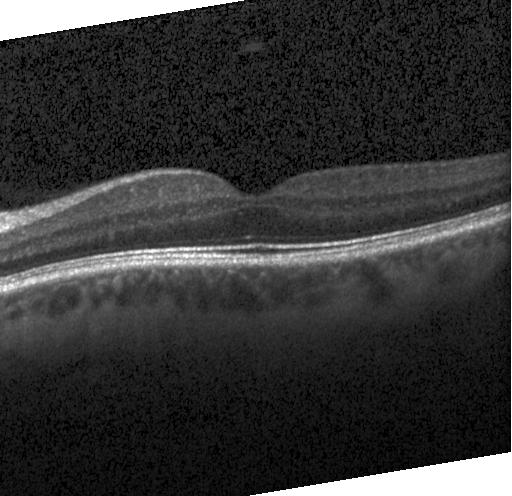

Optical coherence tomography scan — The scan shows no evidence of CNV, DME, or drusen.